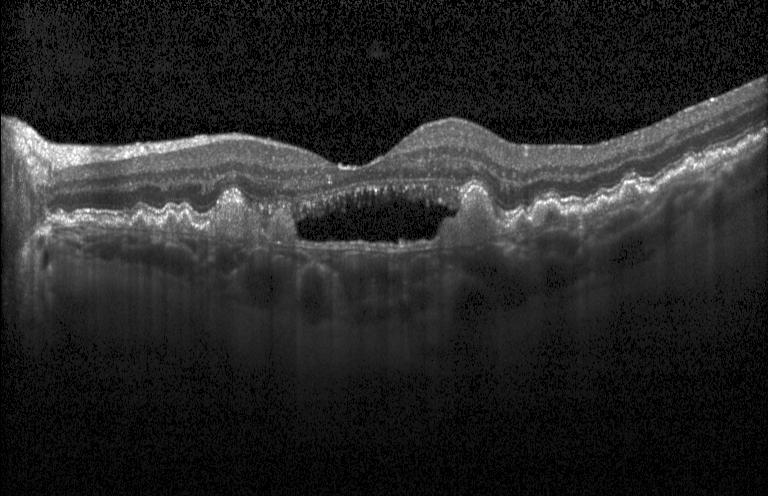

Acquired on a Heidelberg Spectralis. Fovea-centered. SD-OCT. Optical coherence tomography B-scan.
This B-scan demonstrates a choroidal neovascular membrane.